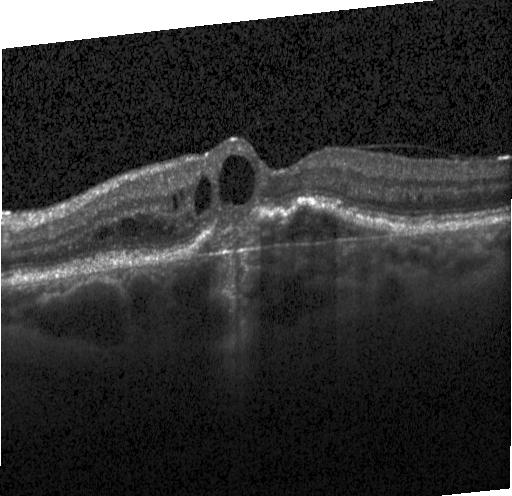 OCT line scan; spectral-domain OCT. Diagnosis: a choroidal neovascular membrane.